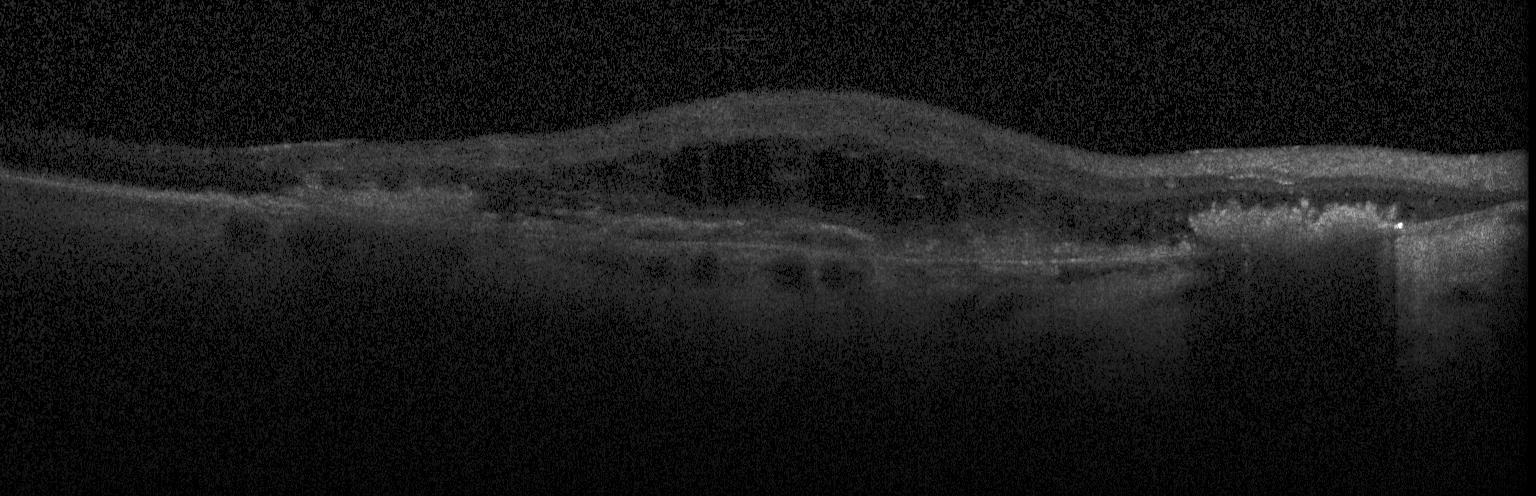
Assessment: a choroidal neovascular membrane.